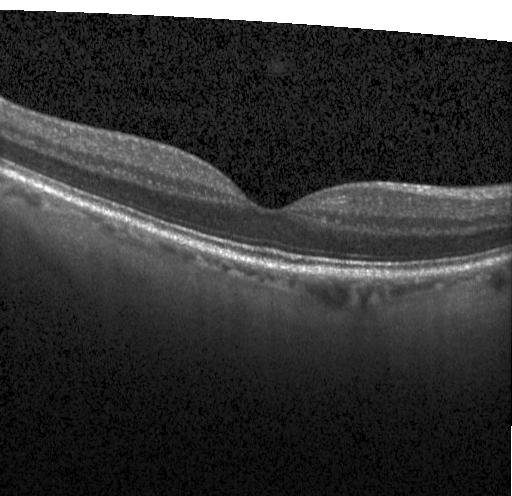 OCT line scan, Heidelberg Spectralis OCT system
Assessment: neither CNV, DME, nor drusen.